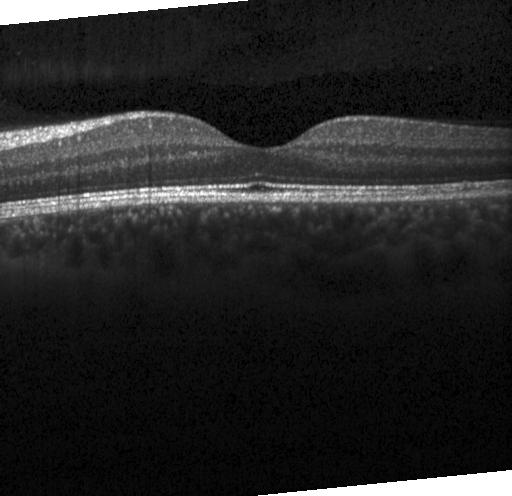
Horizontal scan through the fovea, Heidelberg Spectralis OCT system, optical coherence tomography B-scan — Finding: no evidence of choroidal neovascularization, diabetic macular edema, or drusen.